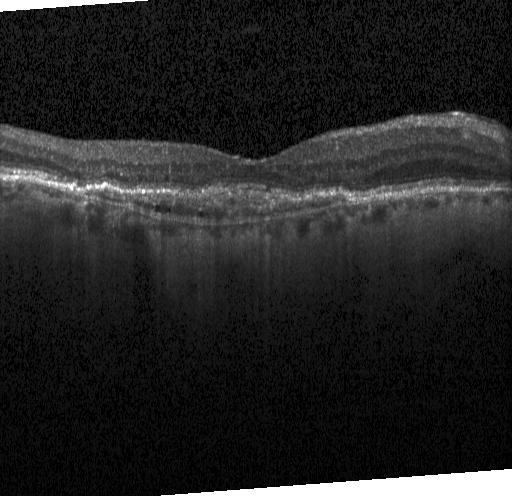
OCT B-scan — Impression: choroidal neovascularization (CNV).